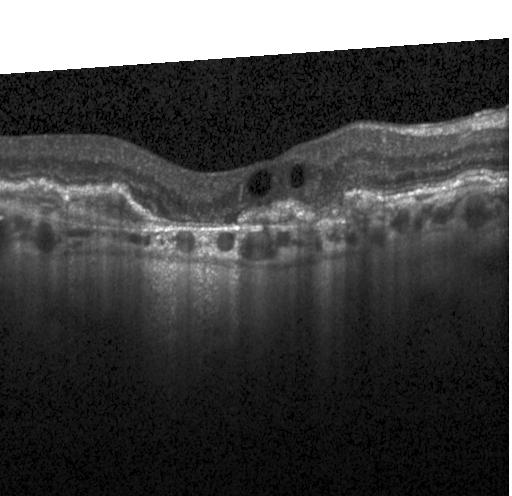 OCT line scan — OCT finding: CNV.